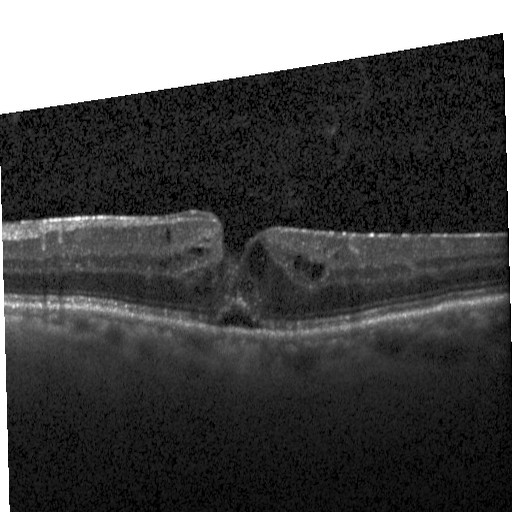 Heidelberg Spectralis, spectral-domain optical coherence tomography, through the macula, OCT B-scan
DME.